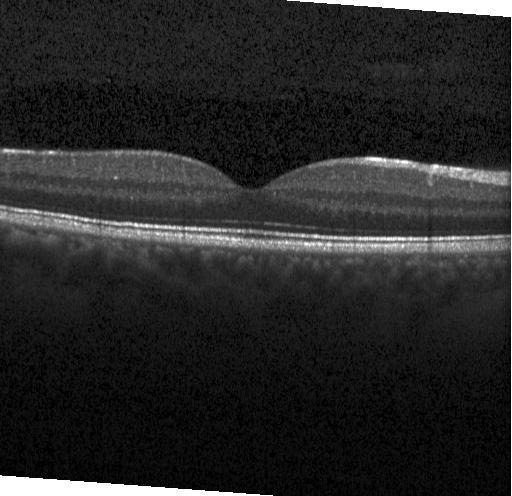

Spectral-domain optical coherence tomography. Optical coherence tomography scan.
OCT finding: neither choroidal neovascularization, diabetic macular edema, nor drusen.